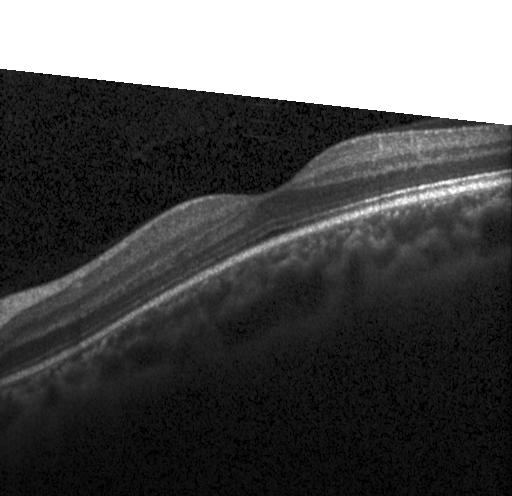

Spectral-domain OCT; retinal OCT B-scan; through the macula; Heidelberg Spectralis OCT system
Impression: no evidence of CNV, DME, or drusen.